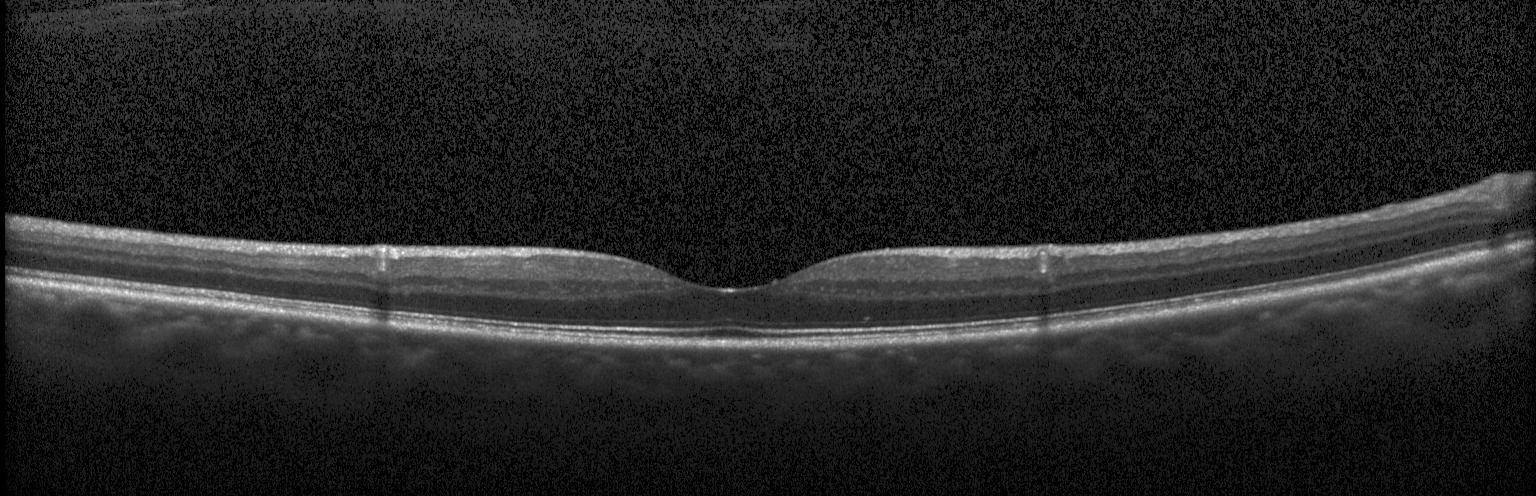
This B-scan demonstrates neither choroidal neovascularization, diabetic macular edema, nor drusen.